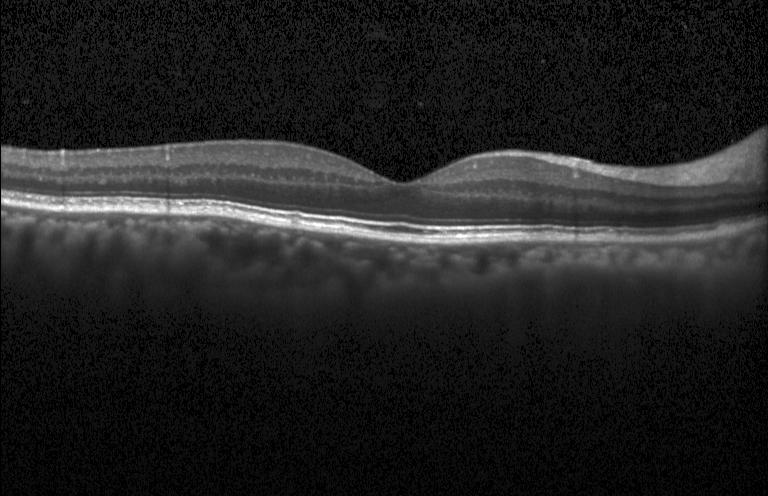
No choroidal neovascularization, diabetic macular edema, or drusen.